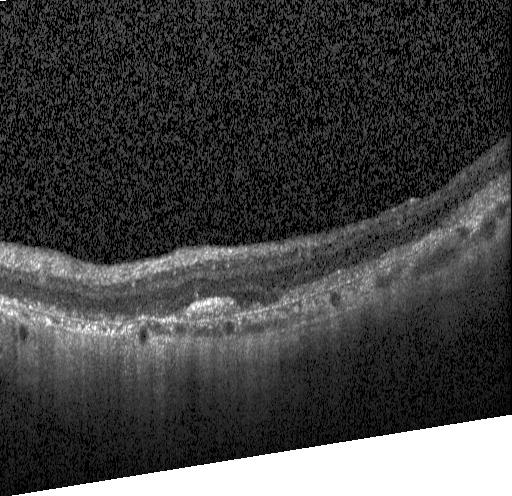

Optical coherence tomography scan — Dx: choroidal neovascularization (CNV).